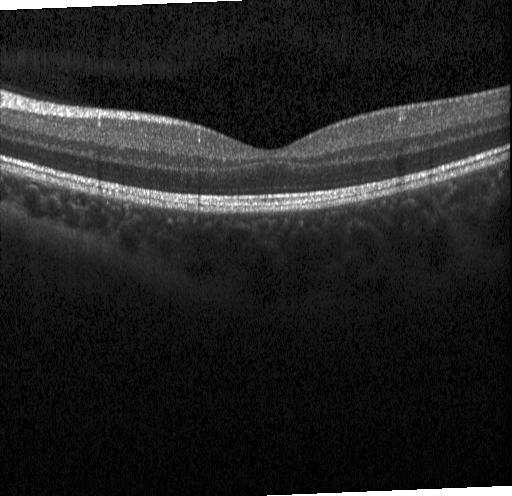 Impression: no CNV, DME, or drusen.